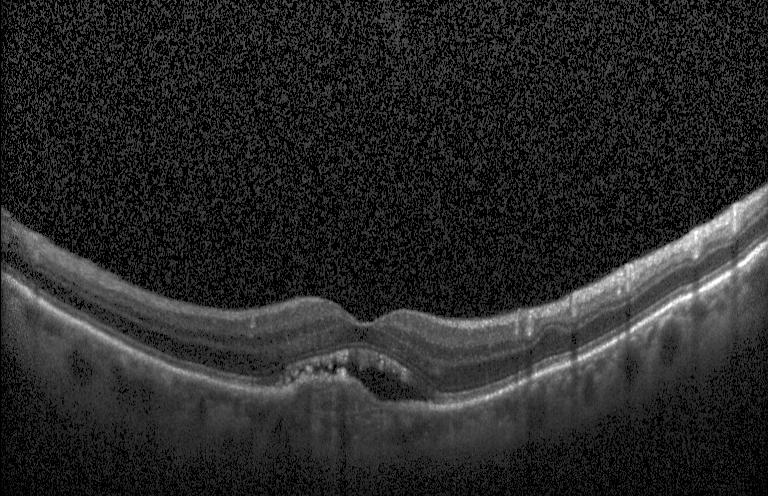 OCT line scan, centered on the fovea, spectral-domain OCT — The scan shows a choroidal neovascular membrane.